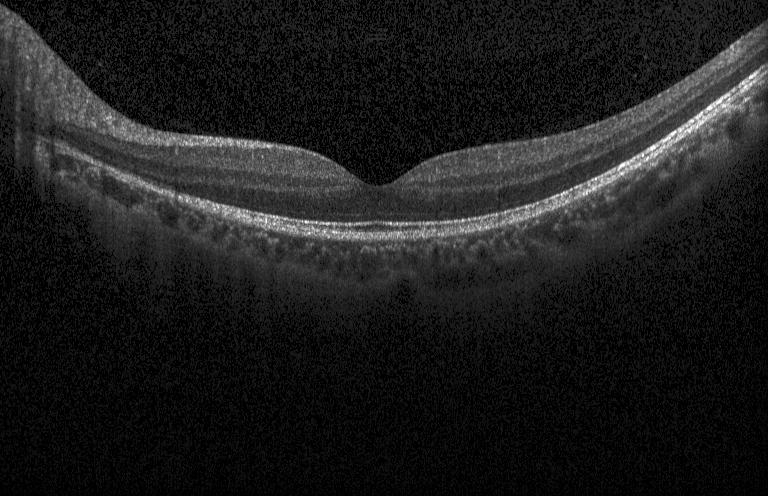

Impression: no evidence of choroidal neovascularization, diabetic macular edema, or drusen.